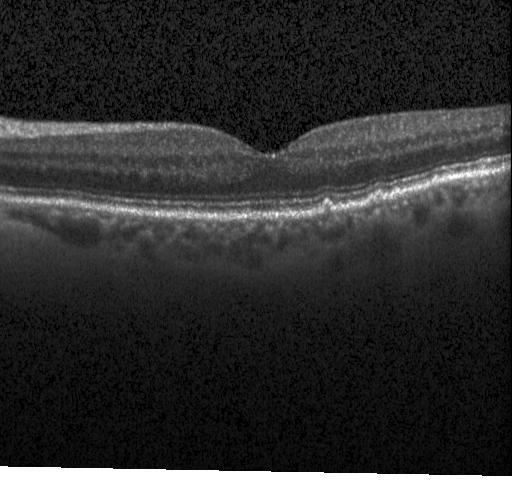
Diagnosis: drusen.